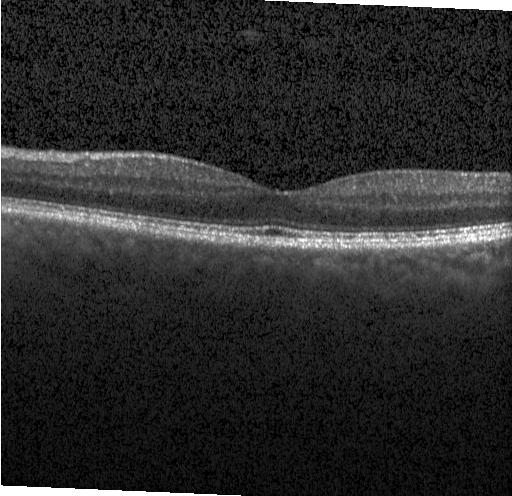 OCT B-scan, macular scan — Dx: neither choroidal neovascularization, diabetic macular edema, nor drusen.